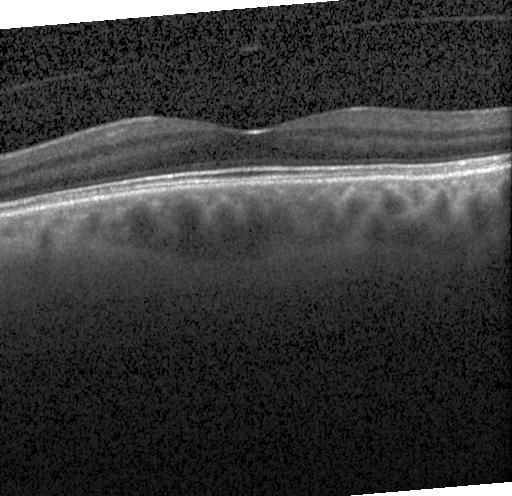
Spectral-domain OCT B-scan: neither CNV, DME, nor drusen.